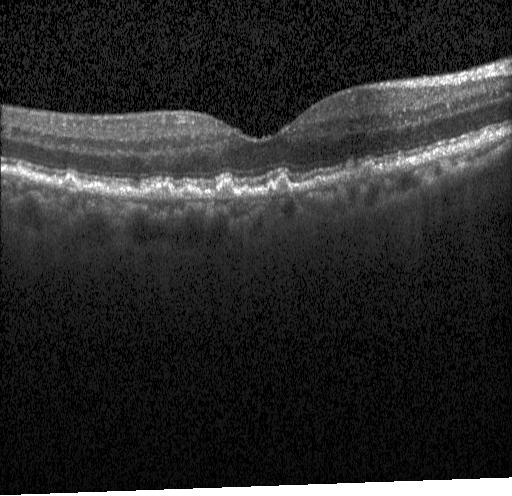 The scan shows sub-RPE drusenoid deposits.